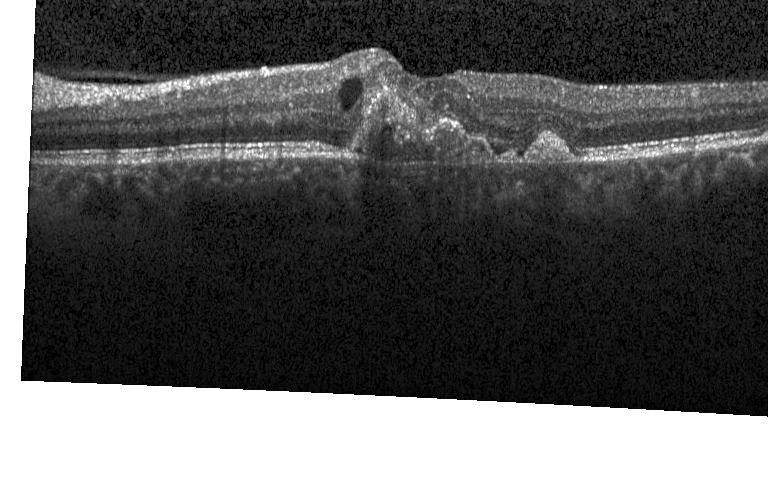
Spectral-domain OCT B-scan: choroidal neovascularization (CNV).